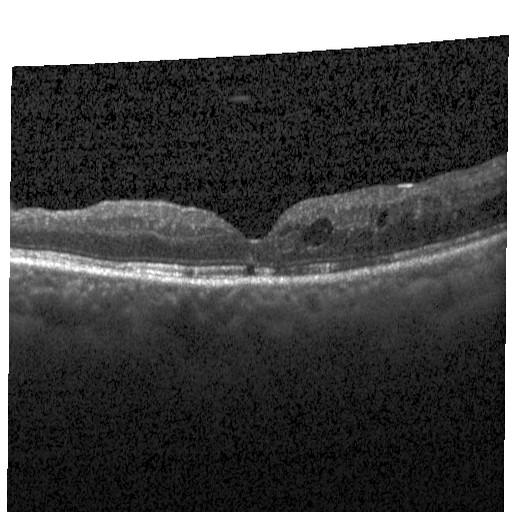

Acquired on a Heidelberg Spectralis · spectral-domain OCT · retinal OCT B-scan · through the macula. This B-scan demonstrates diabetic macular edema.